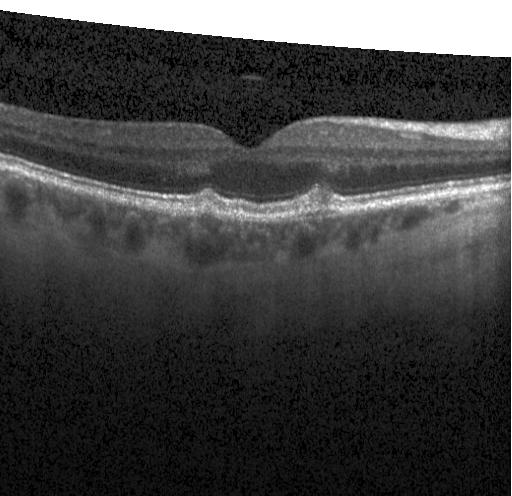

Optical coherence tomography scan.
Assessment: multiple drusen.